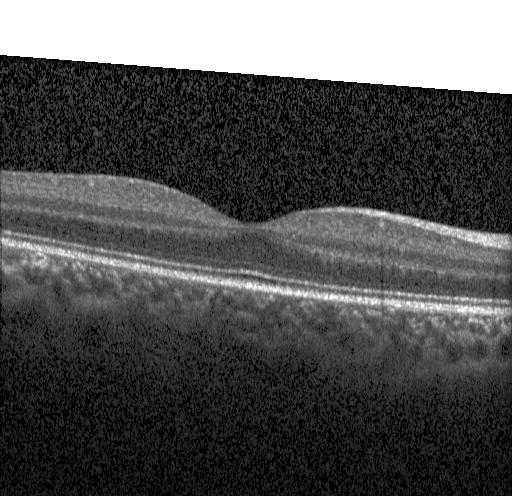

Retinal OCT cross-section — Finding: no choroidal neovascularization, diabetic macular edema, or drusen.